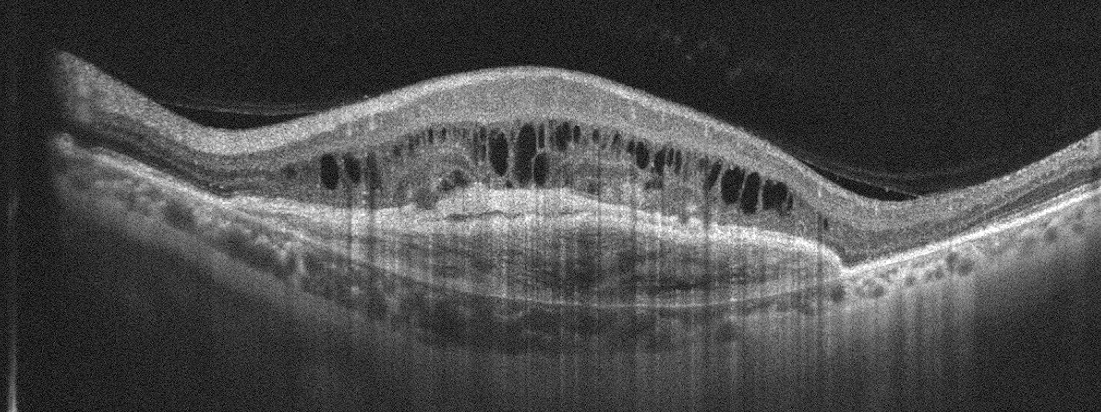

Optovue Avanti RTVue XR. OCT line scan. Through the macula.
Finding: age-related macular degeneration (AMD).